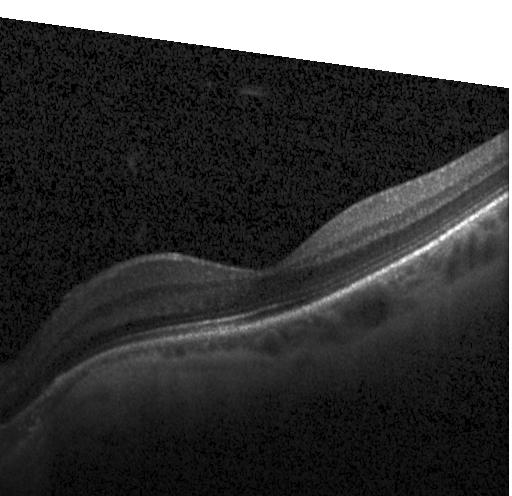 OCT B-scan · Heidelberg Spectralis. Finding: no choroidal neovascularization, no diabetic macular edema, and no drusen.